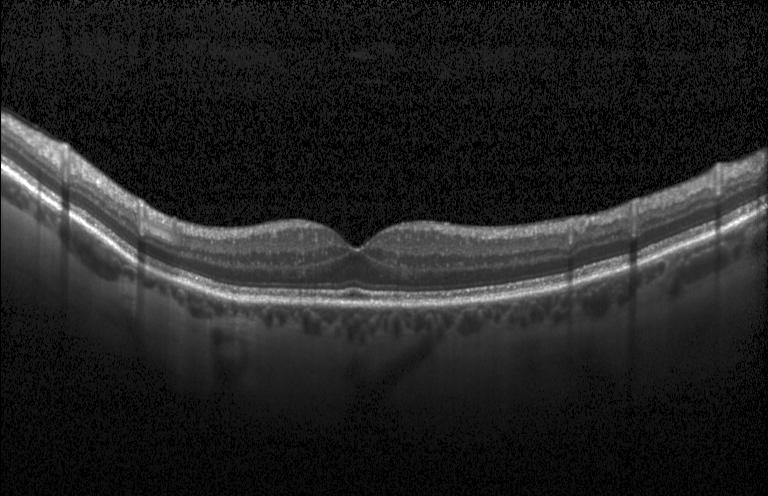
Through the macula; Heidelberg Spectralis OCT system; retinal OCT cross-section; SD-OCT — Diagnosis: no CNV, no DME, and no drusen.